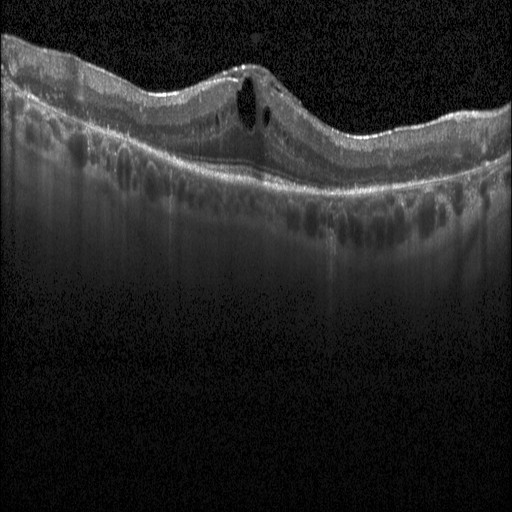
Assessment: diabetic macular edema.